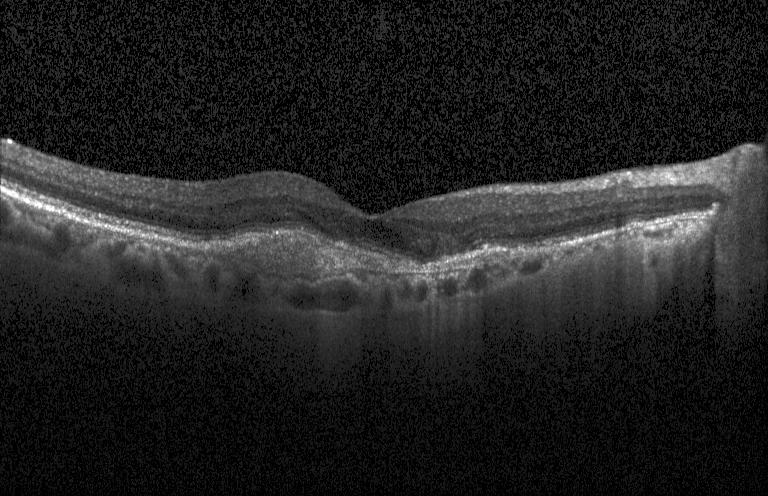

Diagnosis: choroidal neovascularization (CNV).